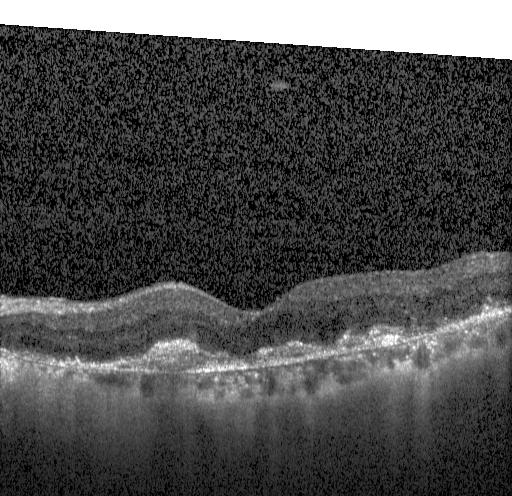

Diagnosis: a choroidal neovascular membrane.